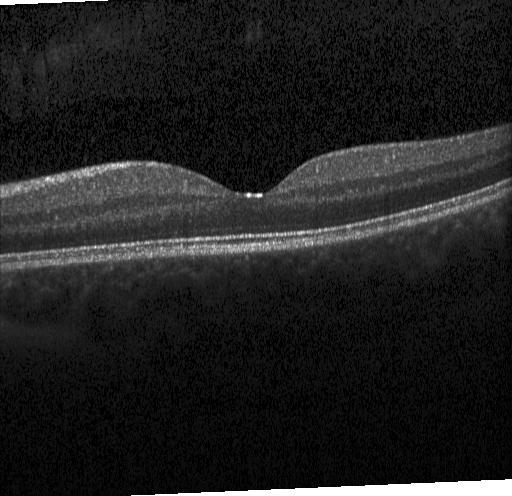
Retinal OCT B-scan. Impression: no CNV, DME, or drusen.